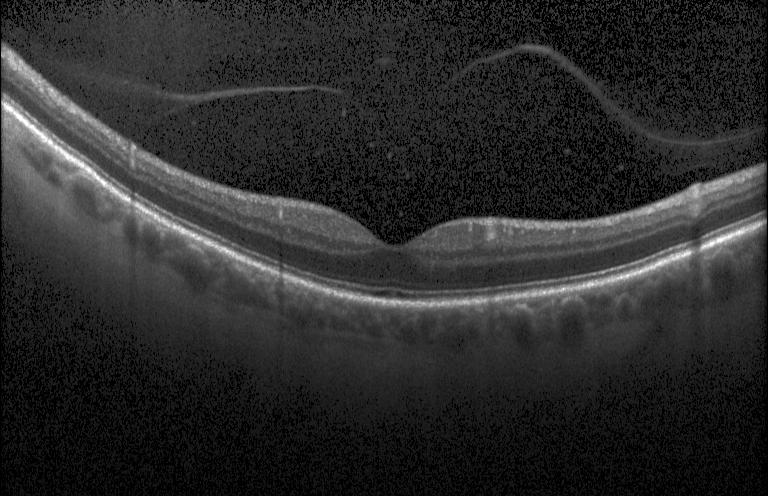

Impression: neither choroidal neovascularization, diabetic macular edema, nor drusen.